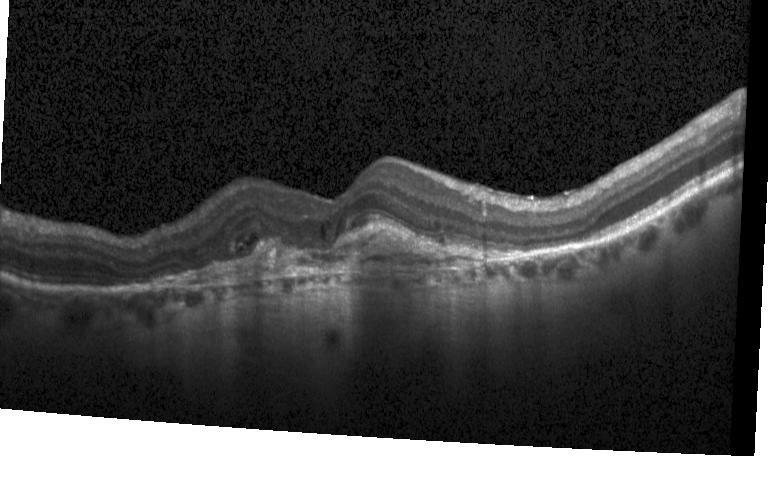

Assessment: a choroidal neovascular membrane.